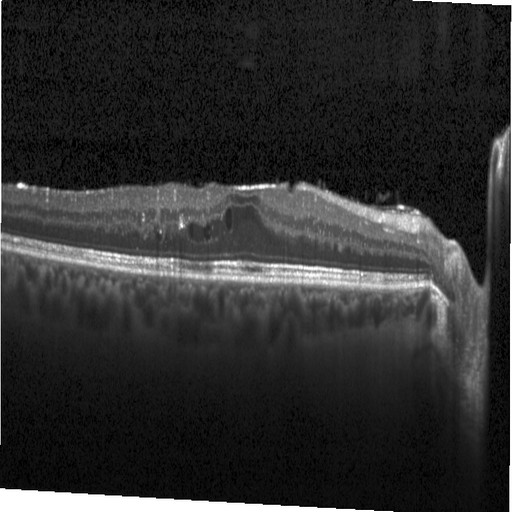
The scan shows diabetic macular edema.